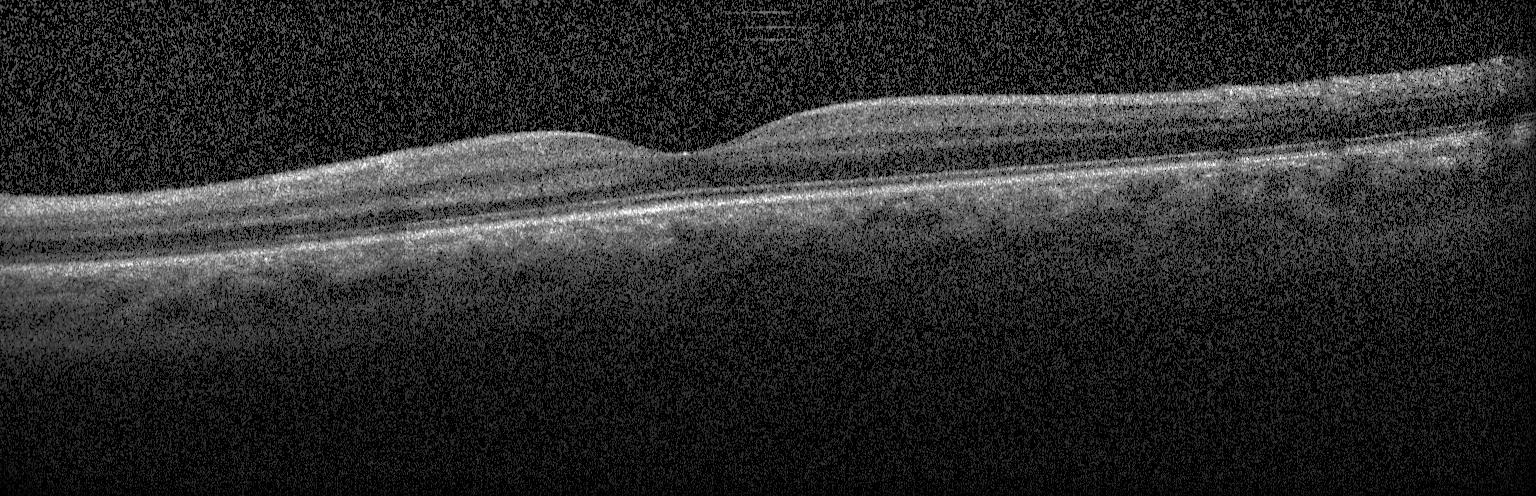
Macular OCT demonstrating neither choroidal neovascularization, diabetic macular edema, nor drusen.